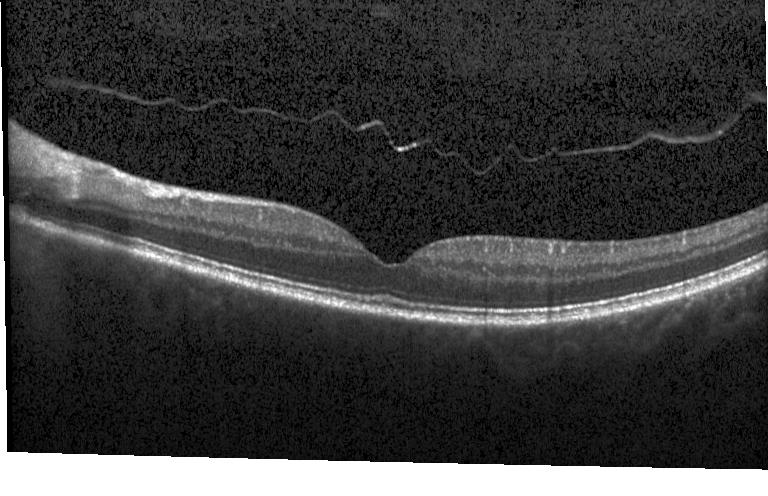

Finding: no CNV, DME, or drusen.